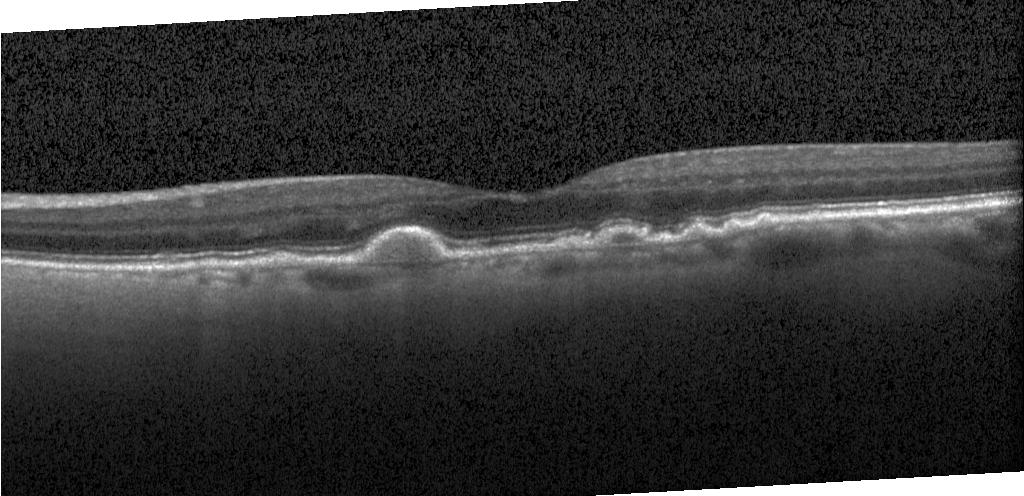 OCT B-scan showing sub-RPE drusenoid deposits.